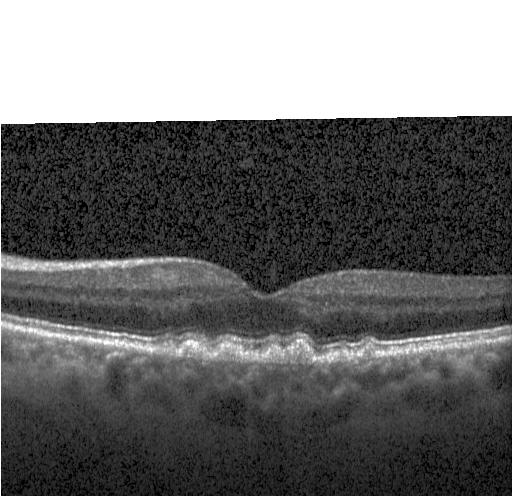

OCT B-scan, Heidelberg Spectralis, SD-OCT.
The scan shows drusen.